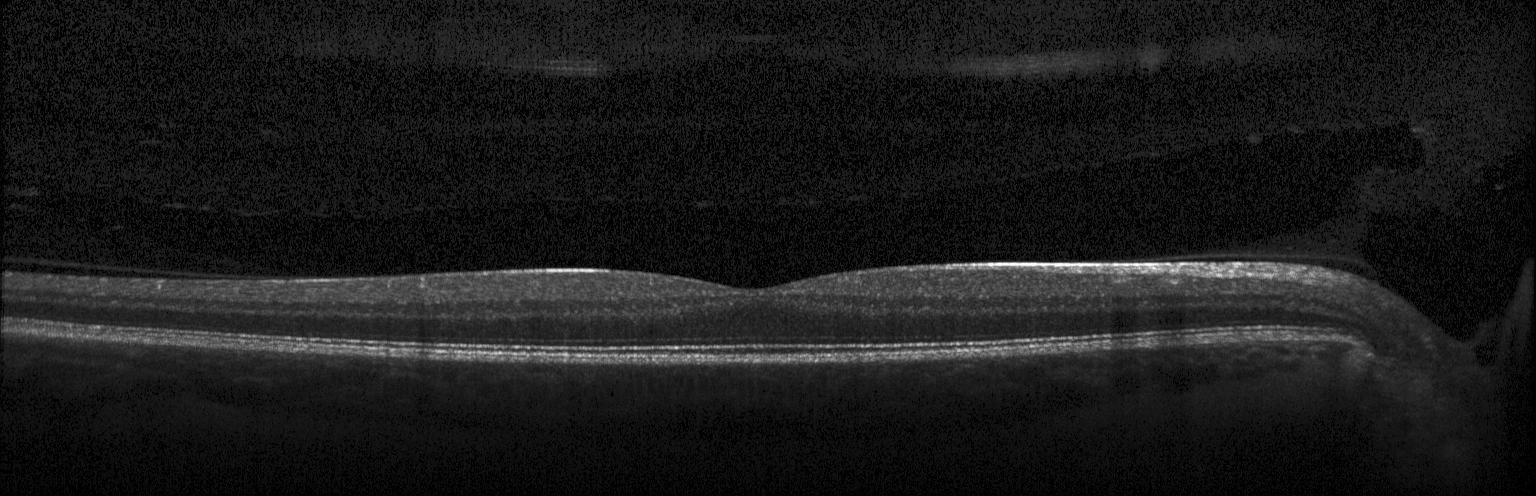
OCT B-scan · through the macula
Impression: no choroidal neovascularization, diabetic macular edema, or drusen.